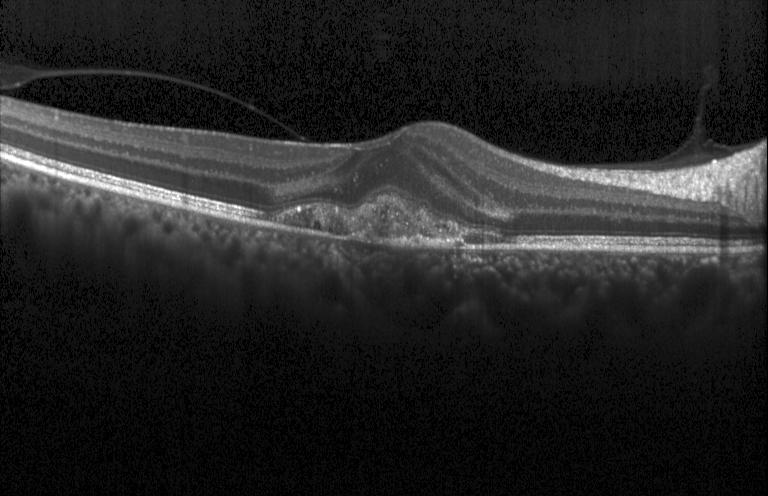

The scan shows choroidal neovascularization.